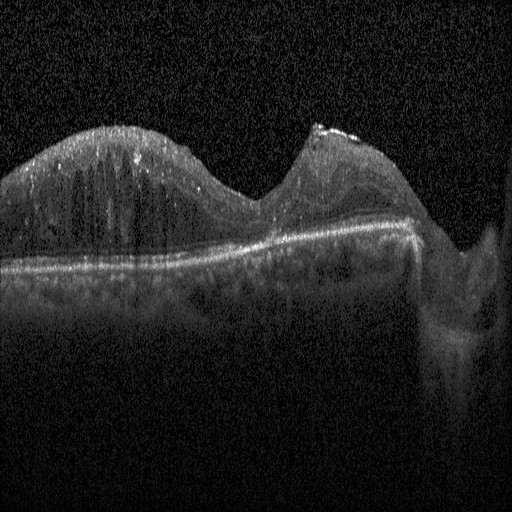 Dx: diabetic macular edema.